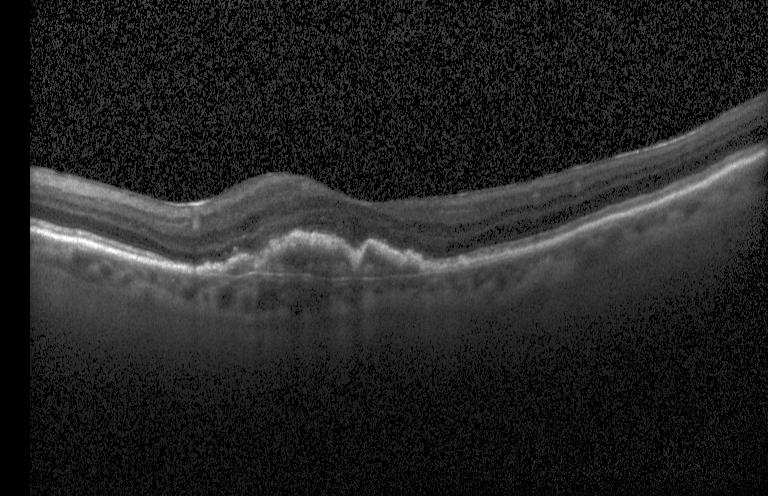 Fovea-centered; OCT line scan. Diagnosis: a choroidal neovascular membrane.